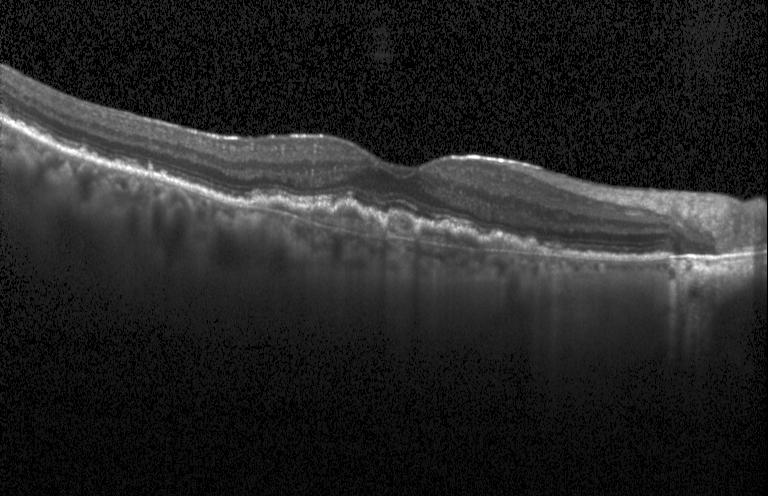 The scan shows CNV.